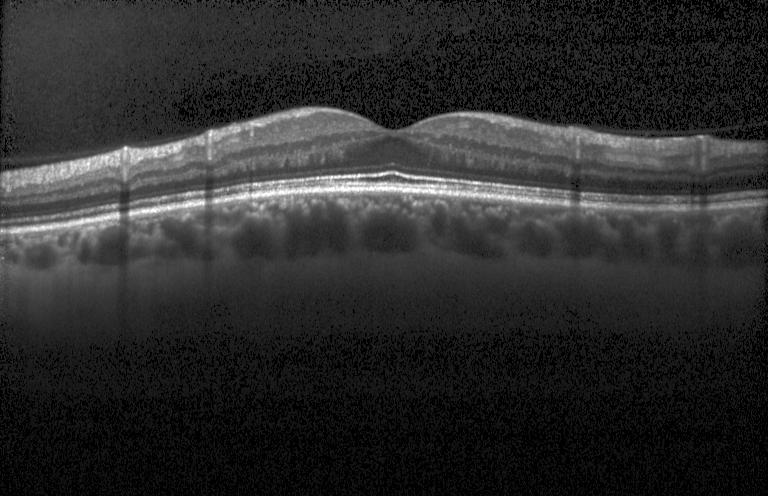

Diagnosis: no evidence of choroidal neovascularization, diabetic macular edema, or drusen.